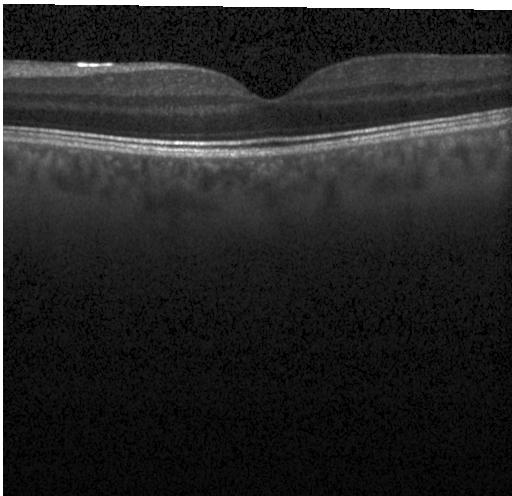 Through the macula, retinal OCT cross-section, spectral-domain optical coherence tomography, instrument: Heidelberg Spectralis. This B-scan demonstrates no CNV, DME, or drusen.